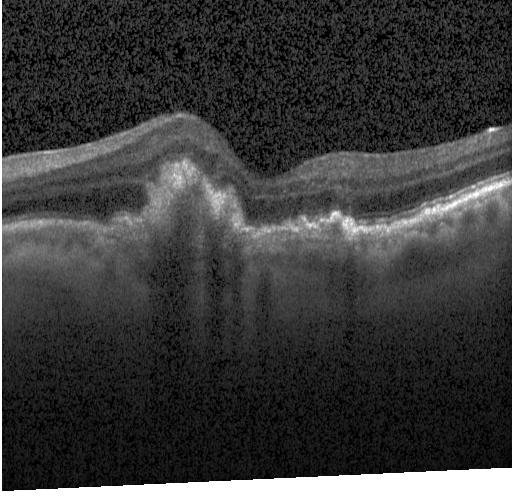 Fovea-centered; OCT line scan. Finding: a choroidal neovascular membrane.